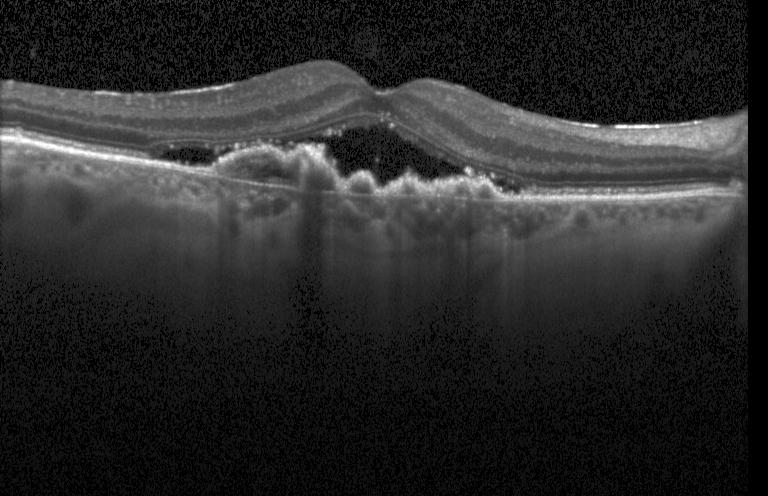 OCT line scan, centered on the fovea, SD-OCT. Assessment: a choroidal neovascular membrane.